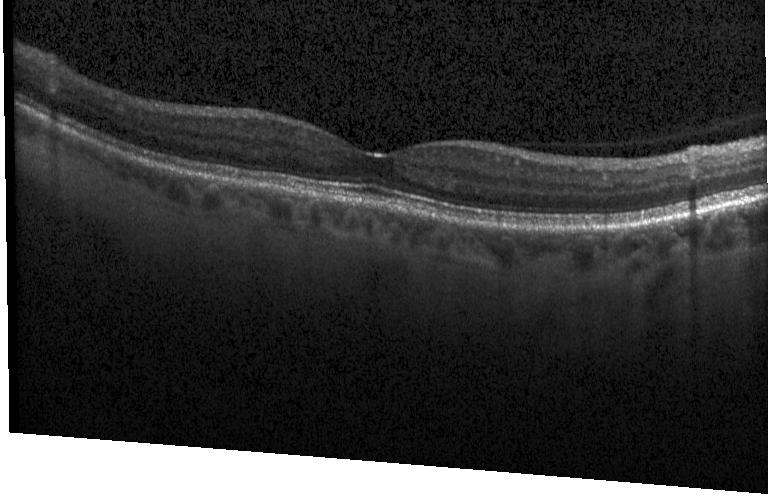
SD-OCT. Fovea-centered. Retinal OCT cross-section. Heidelberg Spectralis OCT system.
Assessment: no choroidal neovascularization, no diabetic macular edema, and no drusen.